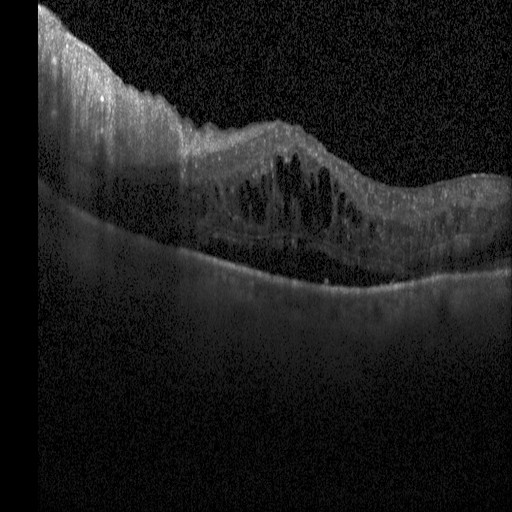

OCT finding: diabetic macular edema.